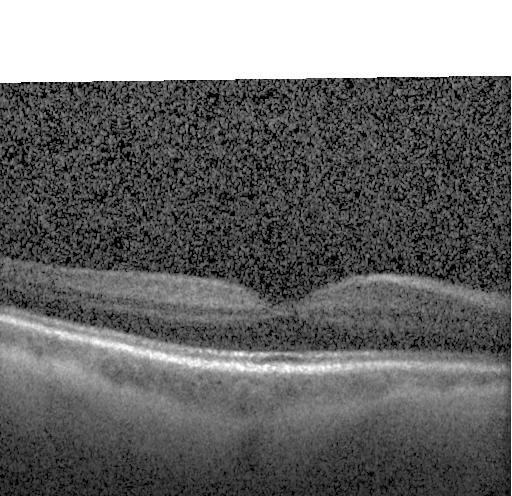

OCT line scan · Heidelberg Spectralis · spectral-domain optical coherence tomography · through the macula — Finding: no choroidal neovascularization, no diabetic macular edema, and no drusen.